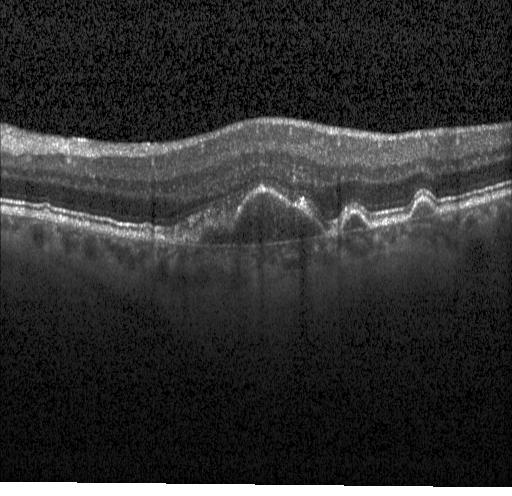

OCT B-scan
Diagnosis: choroidal neovascularization (CNV).